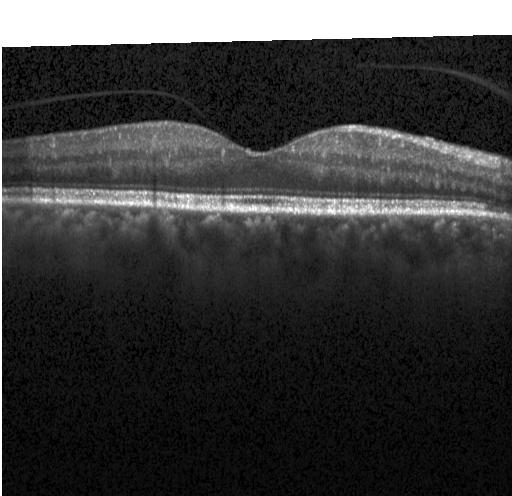
Retinal OCT B-scan. Spectral-domain OCT. Heidelberg Spectralis OCT system
OCT finding: no evidence of CNV, DME, or drusen.